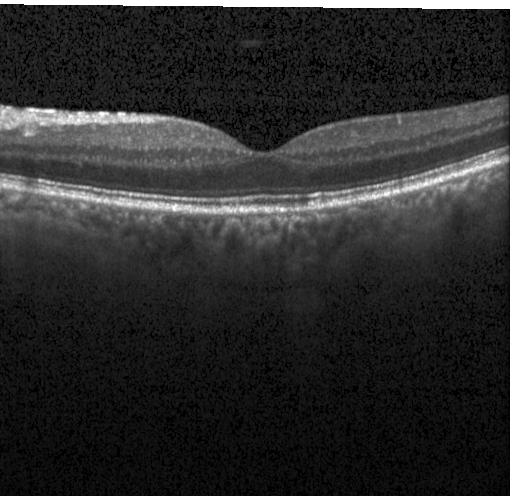 OCT B-scan showing neither choroidal neovascularization, diabetic macular edema, nor drusen.